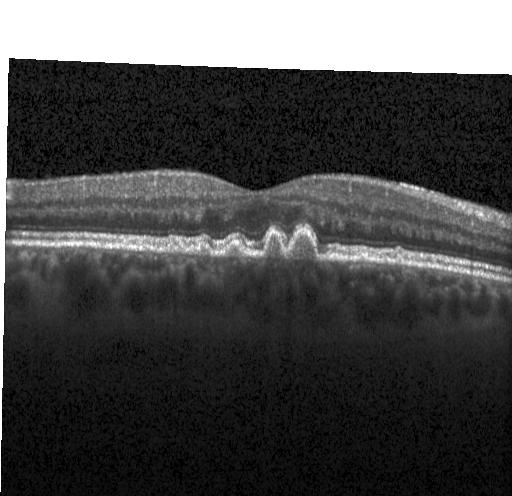

OCT line scan
Macular OCT: sub-RPE drusenoid deposits.